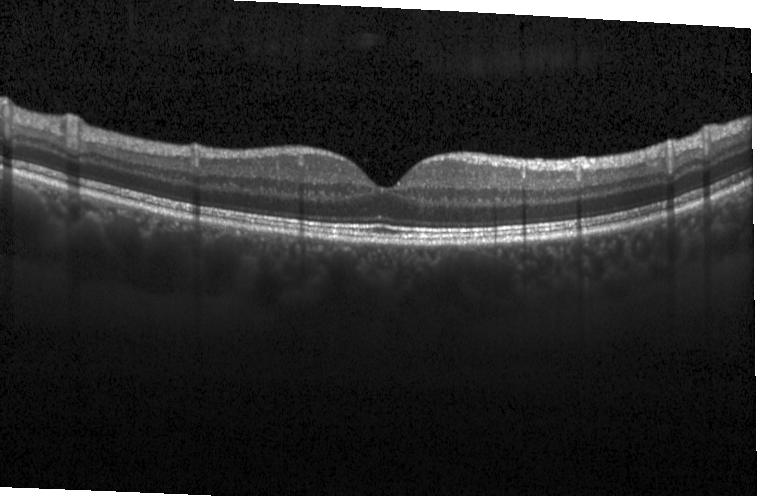 OCT B-scan.
Finding: no evidence of CNV, DME, or drusen.